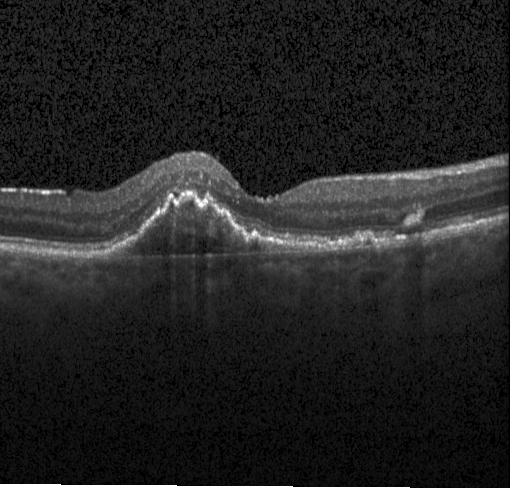

Through the macula, optical coherence tomography B-scan, SD-OCT, instrument: Heidelberg Spectralis. Macular OCT: a choroidal neovascular membrane.